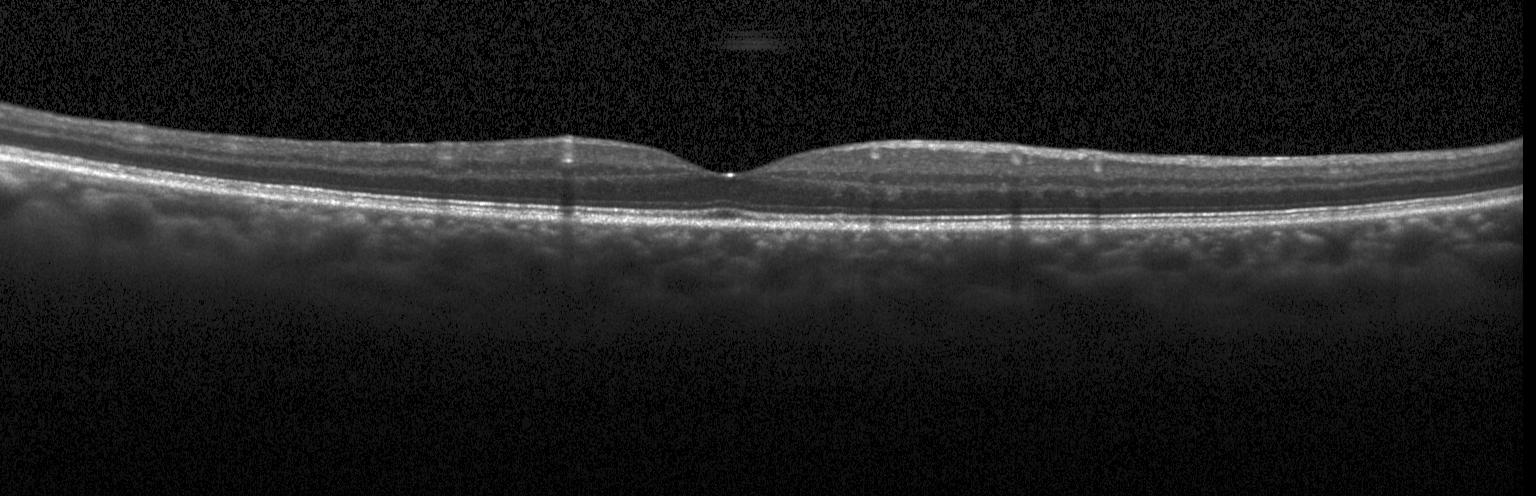 Instrument: Heidelberg Spectralis; optical coherence tomography B-scan; fovea-centered — Diagnosis: no evidence of choroidal neovascularization, diabetic macular edema, or drusen.